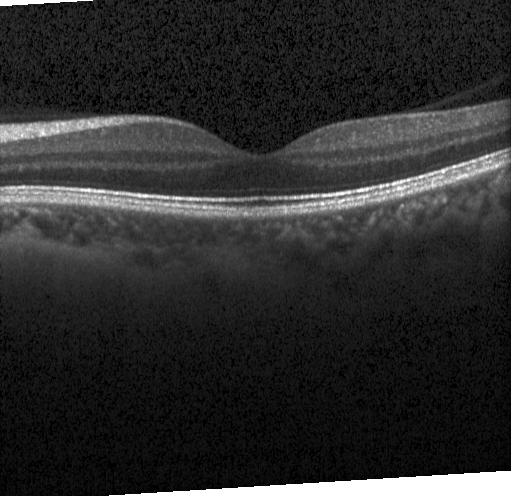 OCT line scan. This B-scan demonstrates no choroidal neovascularization, no diabetic macular edema, and no drusen.